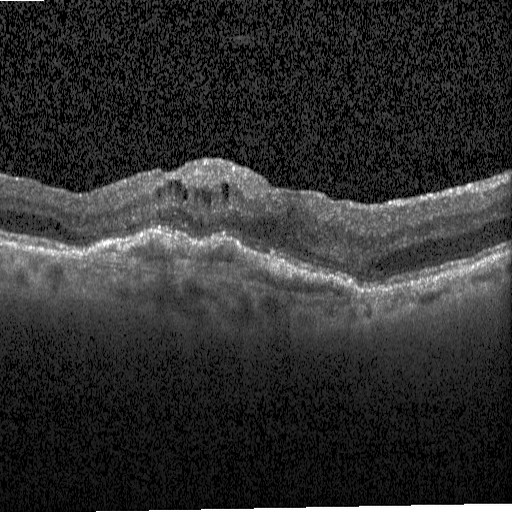 Macular OCT: diabetic macular edema (DME).